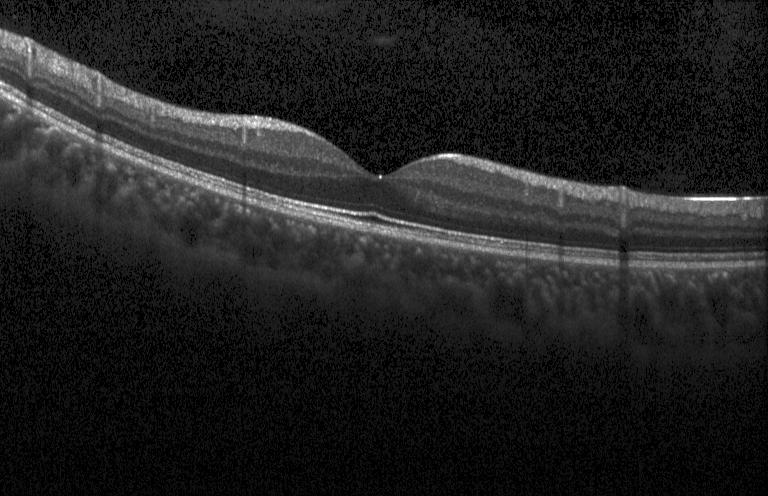 SD-OCT. Fovea-centered. OCT B-scan.
Impression: neither choroidal neovascularization, diabetic macular edema, nor drusen.